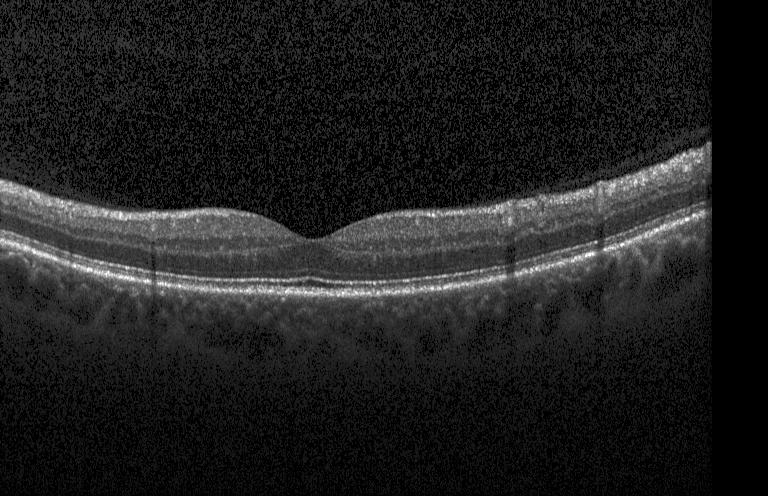
Optical coherence tomography B-scan. Macular scan
The scan shows neither choroidal neovascularization, diabetic macular edema, nor drusen.